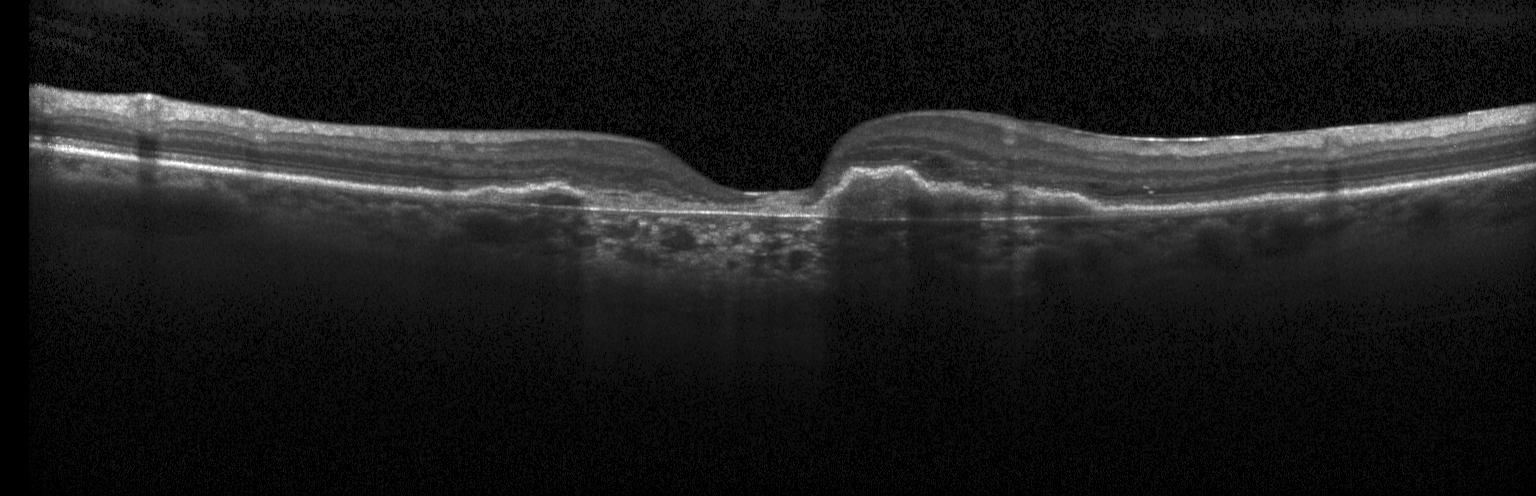

OCT line scan · macular scan — Diagnosis: a choroidal neovascular membrane.